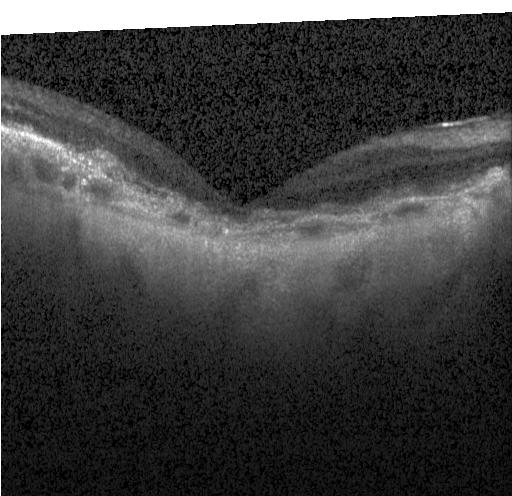 Finding: a choroidal neovascular membrane.